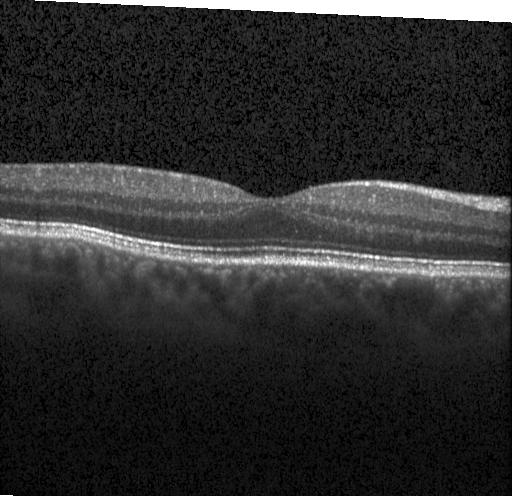
Macular OCT: neither choroidal neovascularization, diabetic macular edema, nor drusen.